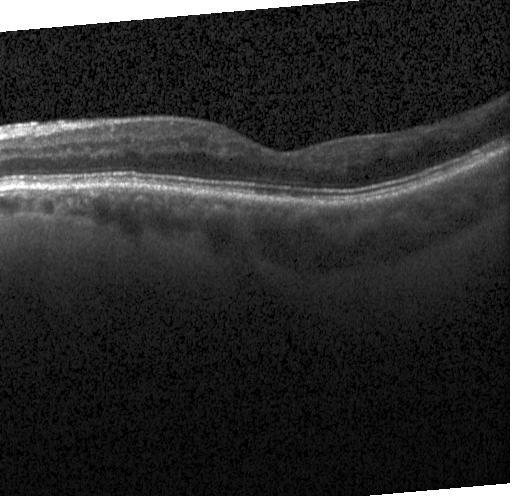 Finding: no CNV, DME, or drusen.